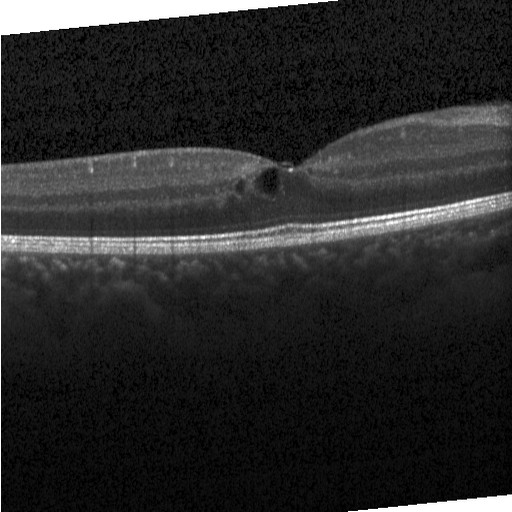
OCT B-scan. Macular scan.
OCT finding: DME.